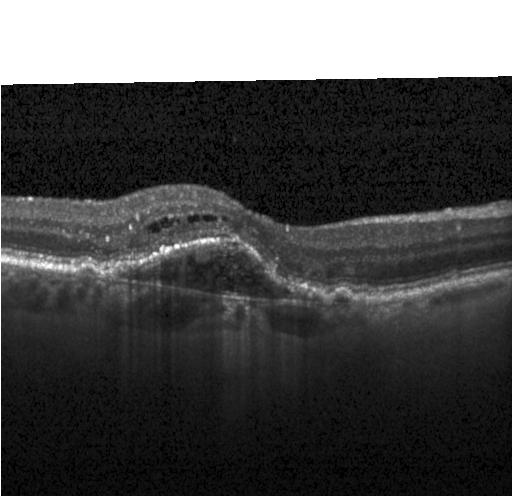

Spectral-domain OCT B-scan: choroidal neovascularization.